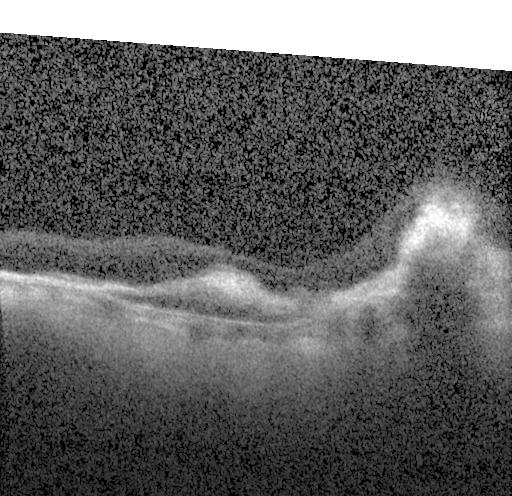

SD-OCT. Retinal OCT B-scan — Assessment: a choroidal neovascular membrane.